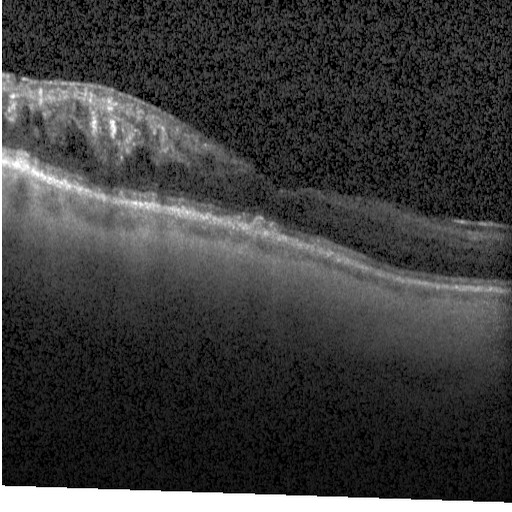 Optical coherence tomography scan; acquired on a Heidelberg Spectralis
Diabetic macular edema.